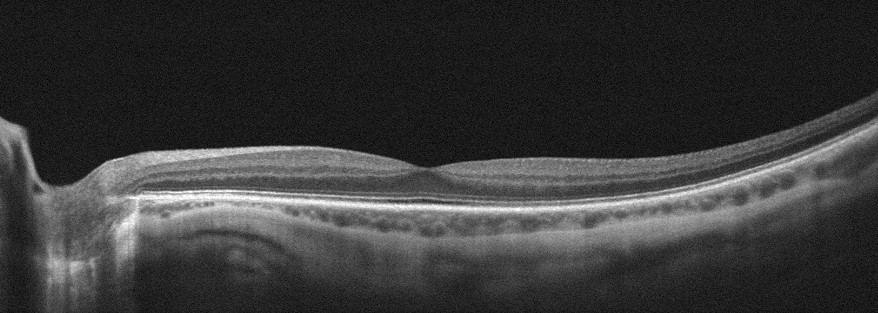
Optical coherence tomography B-scan. Instrument: Optovue Avanti RTVue XR. Macular scan. Finding: no AMD, DME, ERM, RAO, RVO, or VID.